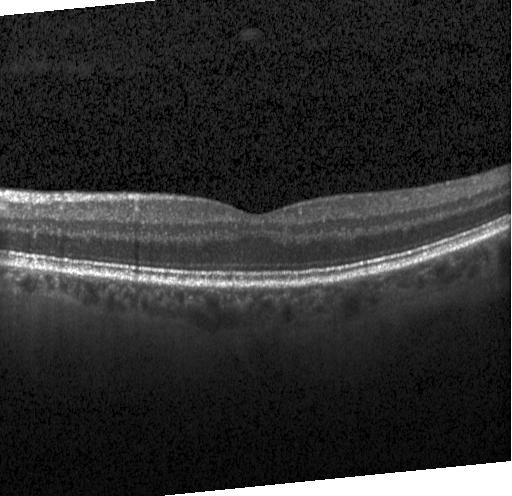

OCT B-scan, spectral-domain OCT, acquired on a Heidelberg Spectralis, centered on the fovea.
OCT finding: no choroidal neovascularization, no diabetic macular edema, and no drusen.